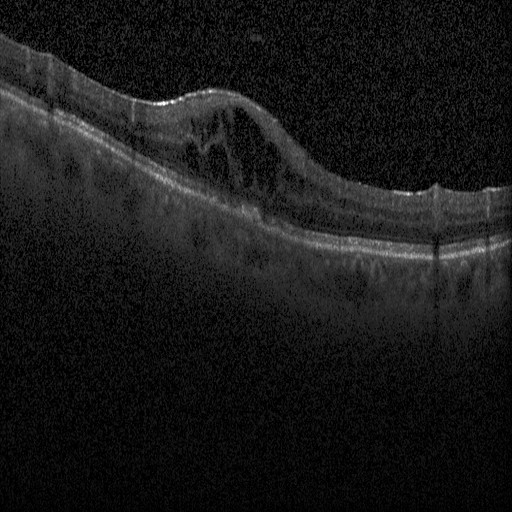
OCT line scan.
Diagnosis: diabetic macular edema (DME).